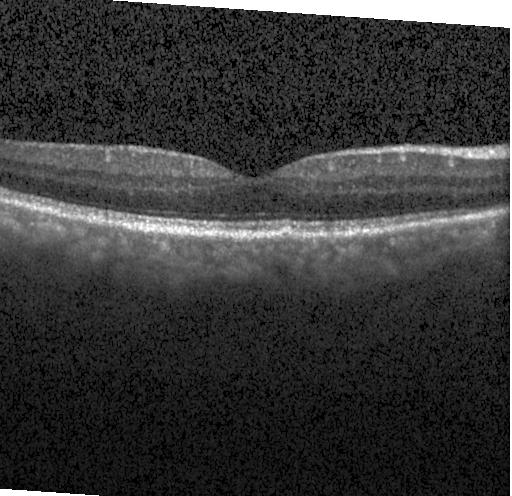 Acquired on a Heidelberg Spectralis. OCT B-scan. Spectral-domain optical coherence tomography. Macular scan.
This B-scan demonstrates no evidence of choroidal neovascularization, diabetic macular edema, or drusen.